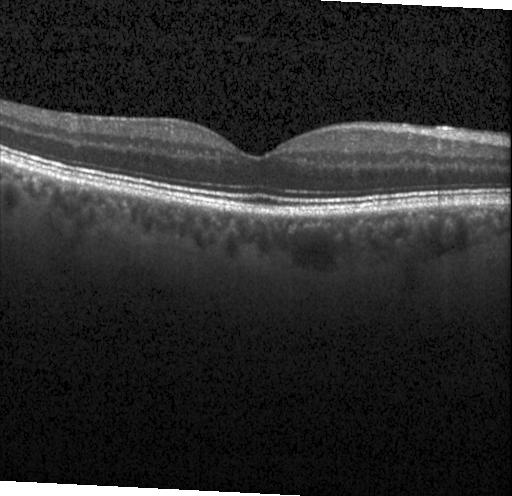 Retinal OCT B-scan.
Finding: neither choroidal neovascularization, diabetic macular edema, nor drusen.